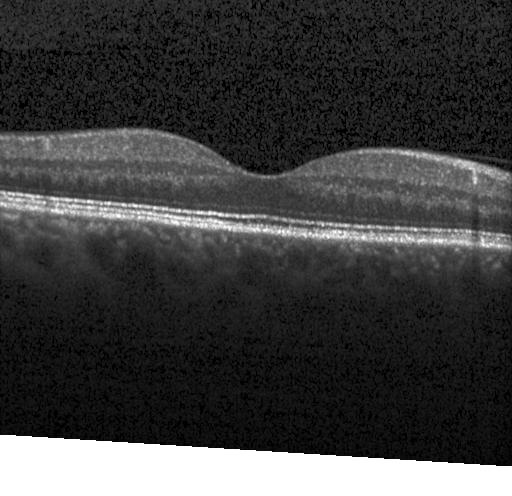

Macular scan · OCT B-scan. Finding: no evidence of choroidal neovascularization, diabetic macular edema, or drusen.